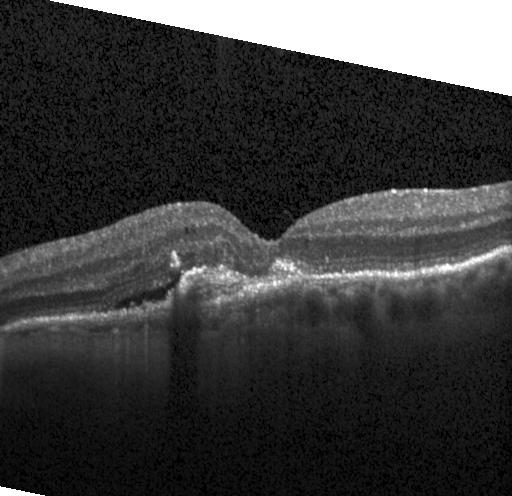

Retinal OCT B-scan; spectral-domain OCT; instrument: Heidelberg Spectralis; horizontal scan through the fovea
Finding: a choroidal neovascular membrane.